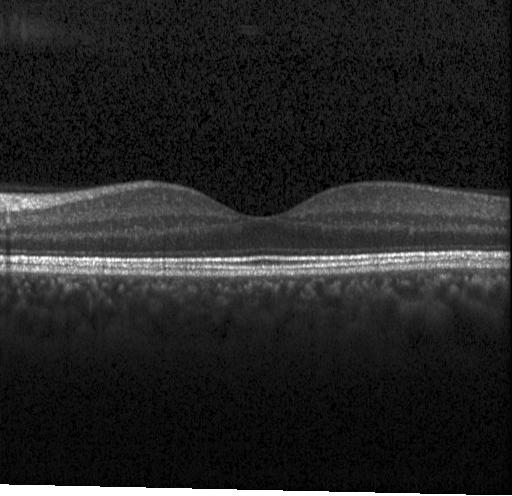 This B-scan demonstrates no choroidal neovascularization, diabetic macular edema, or drusen.